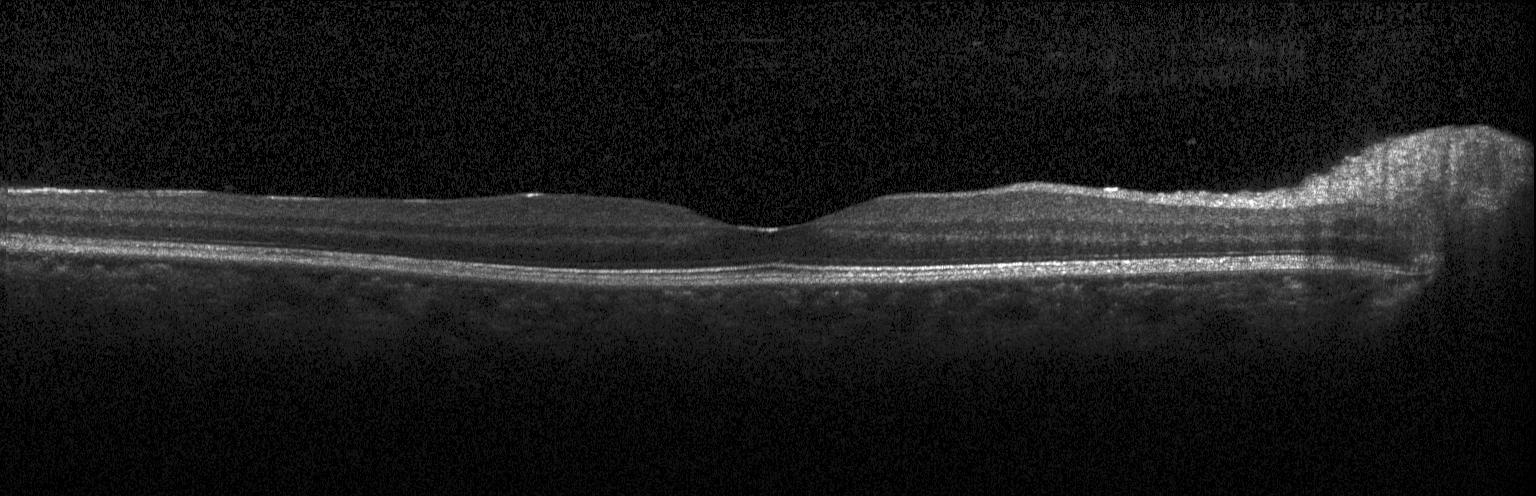 OCT scan showing neither choroidal neovascularization, diabetic macular edema, nor drusen.